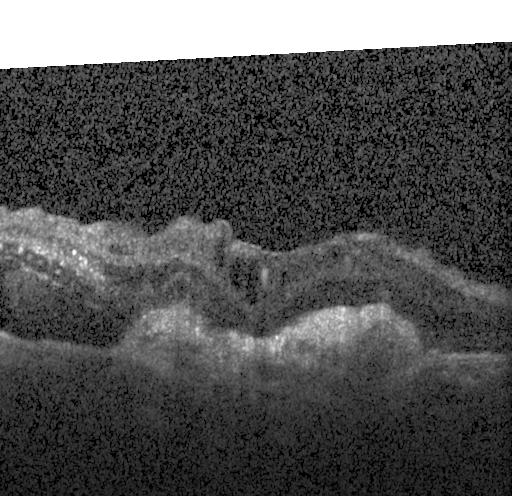

Retinal OCT cross-section showing CNV.